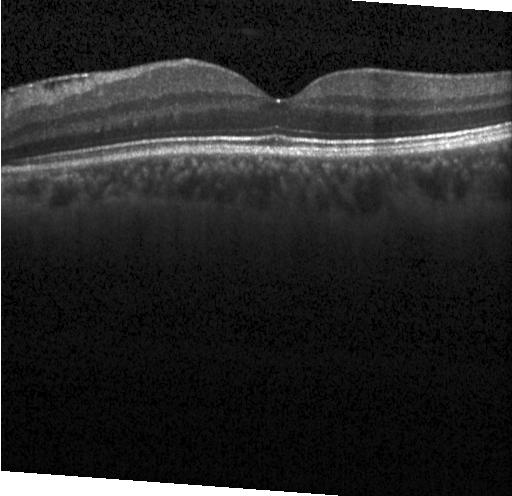 Spectral-domain OCT, centered on the fovea, OCT B-scan, Heidelberg Spectralis — OCT finding: no evidence of choroidal neovascularization, diabetic macular edema, or drusen.